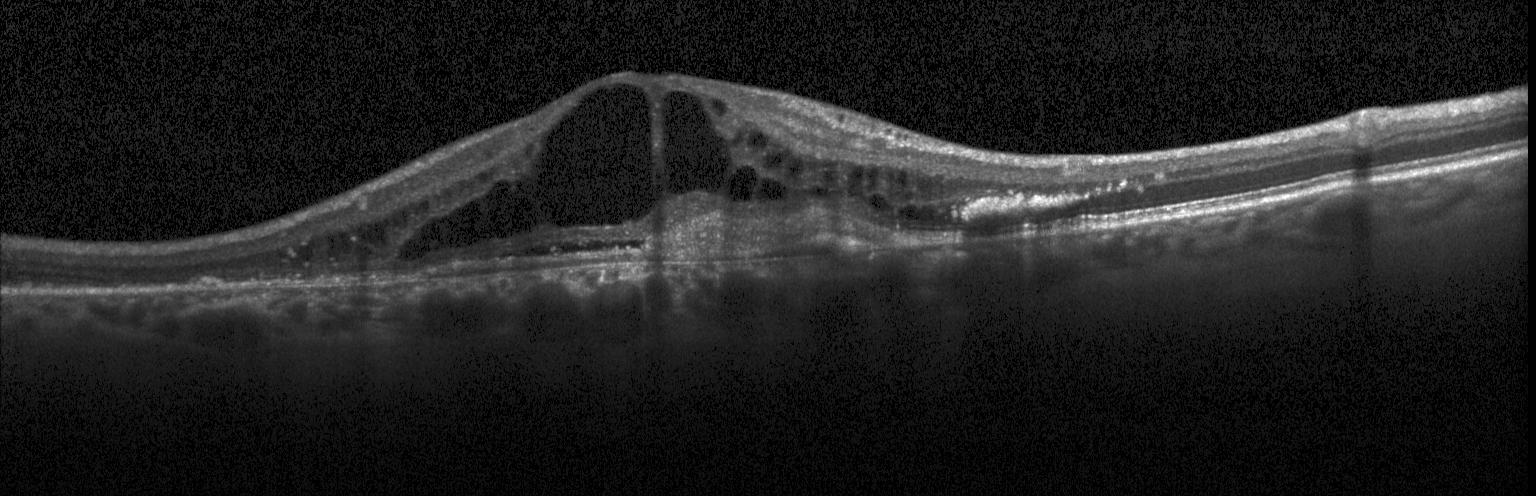
Heidelberg Spectralis OCT system, OCT B-scan, spectral-domain optical coherence tomography — OCT finding: choroidal neovascularization.